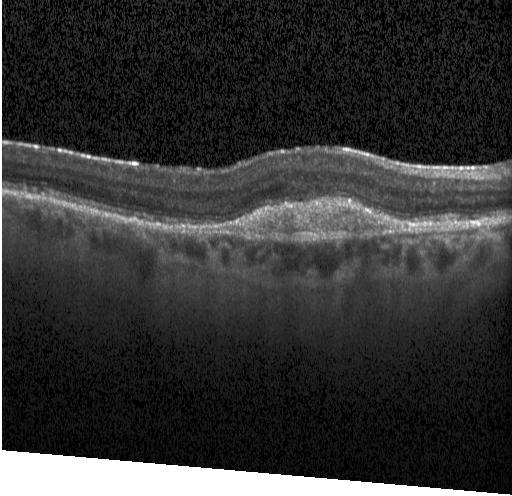
OCT line scan
Diagnosis: choroidal neovascularization (CNV).